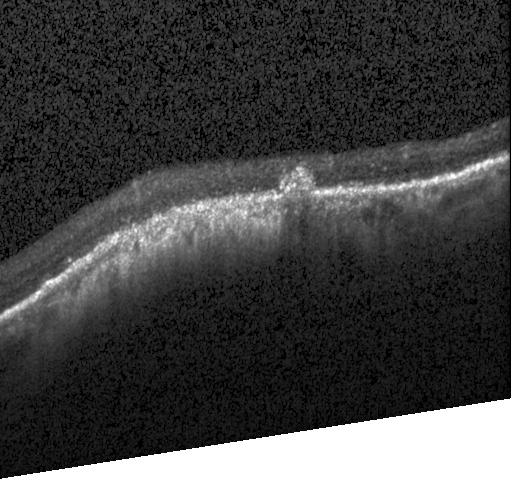

This B-scan demonstrates choroidal neovascularization.